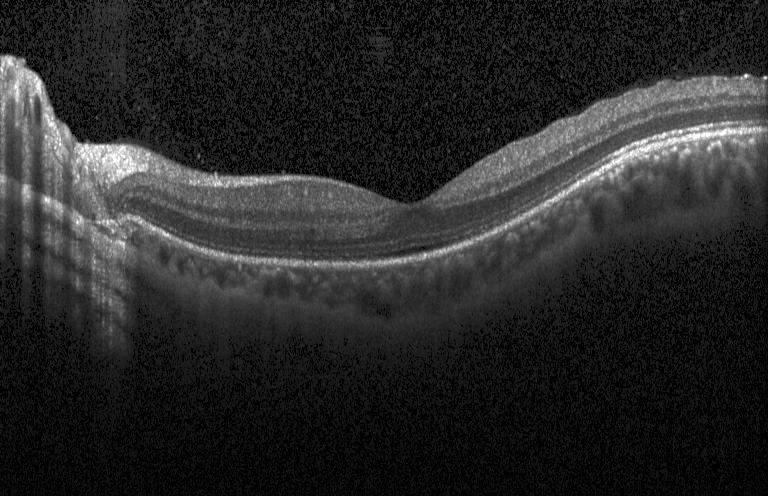

Optical coherence tomography B-scan; through the macula — Neither CNV, DME, nor drusen.